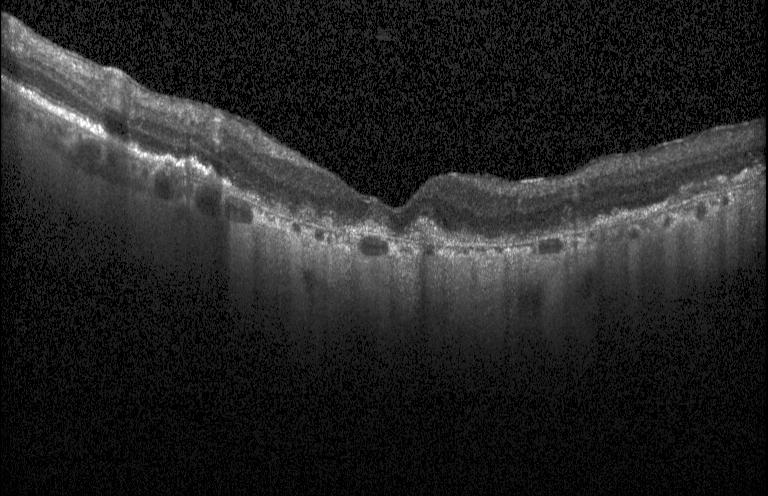 Optical coherence tomography B-scan.
This B-scan demonstrates CNV.